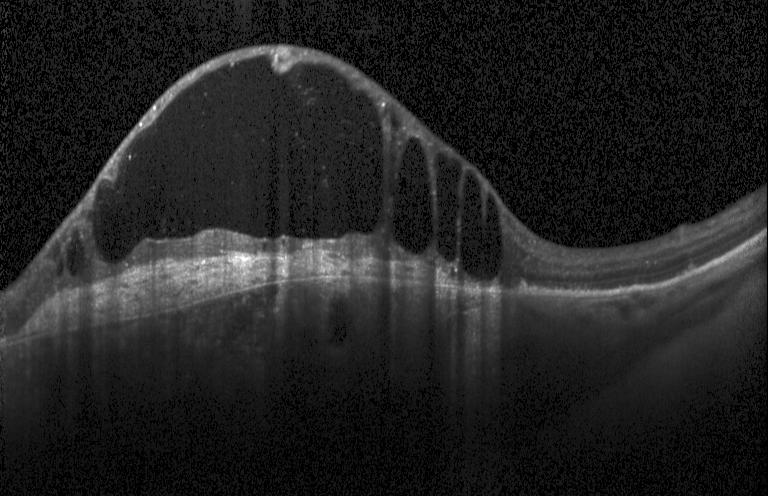
Retinal OCT cross-section showing choroidal neovascularization (CNV).